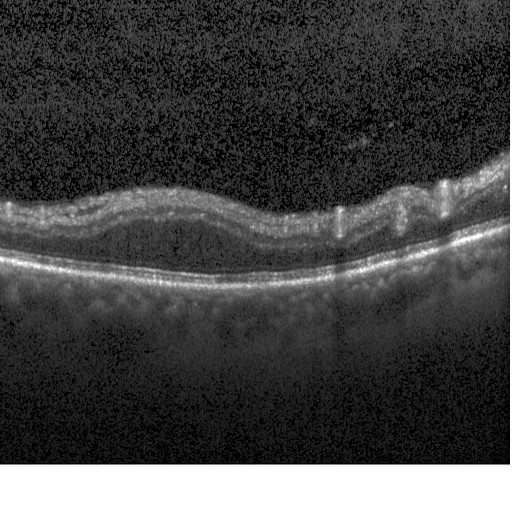

The scan shows diabetic macular edema.